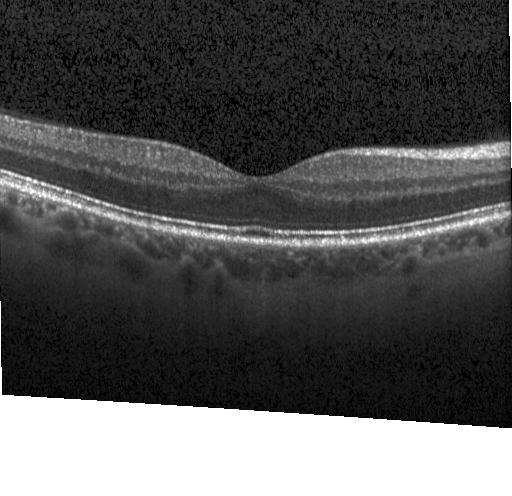 Diagnosis: no CNV, no DME, and no drusen.